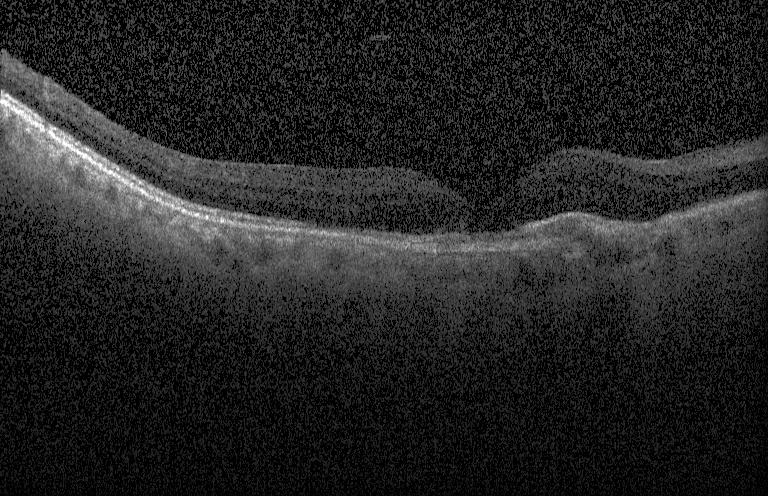 Macular OCT demonstrating a choroidal neovascular membrane.